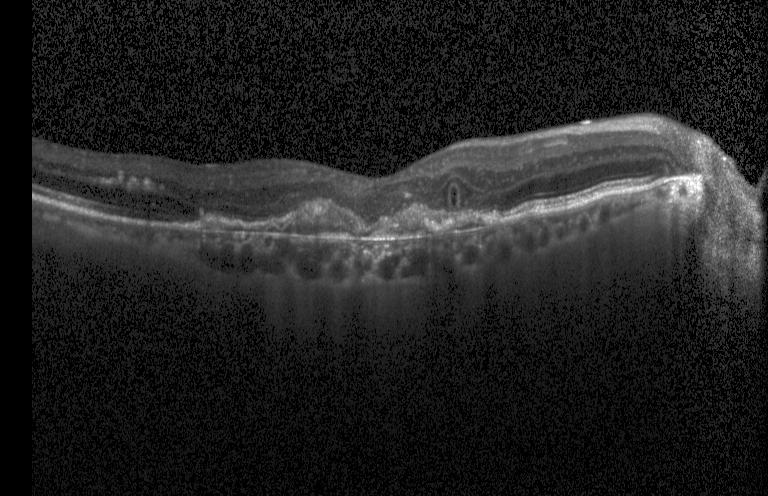

A choroidal neovascular membrane.